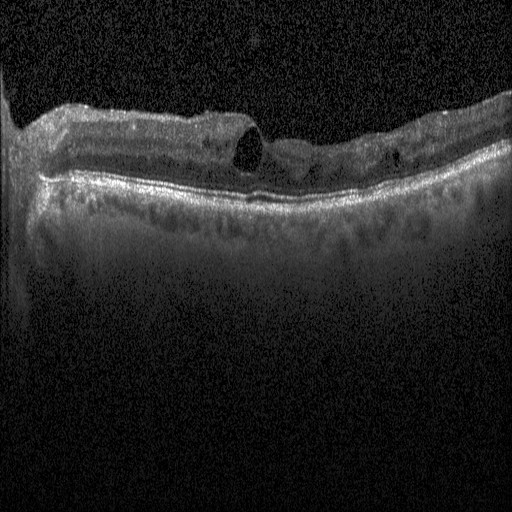

Macular OCT: diabetic macular edema (DME).